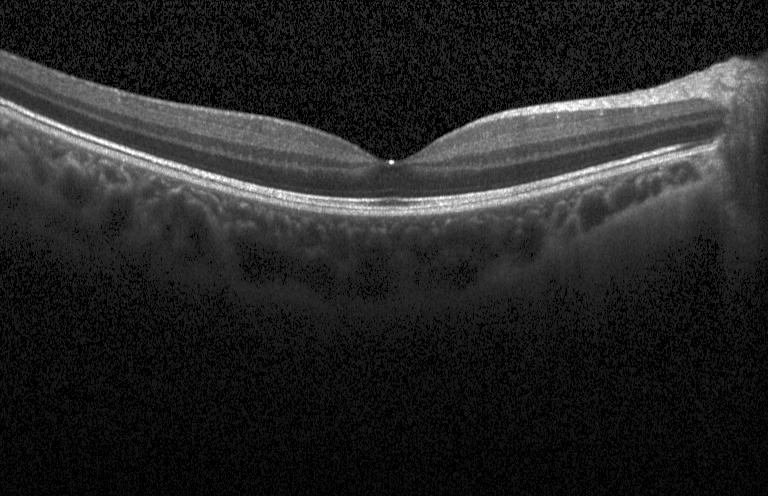

Finding: no choroidal neovascularization, no diabetic macular edema, and no drusen.